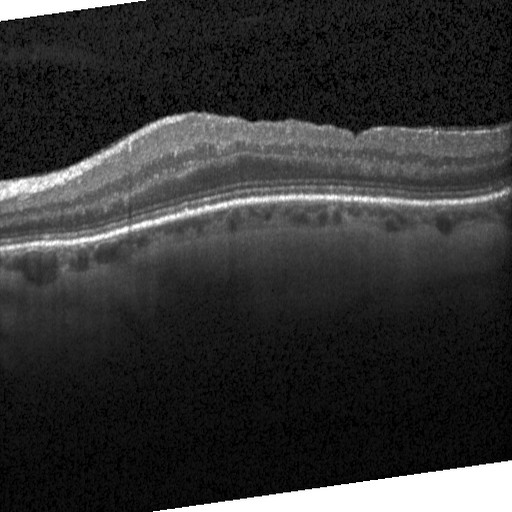
Dx: diabetic macular edema (DME).